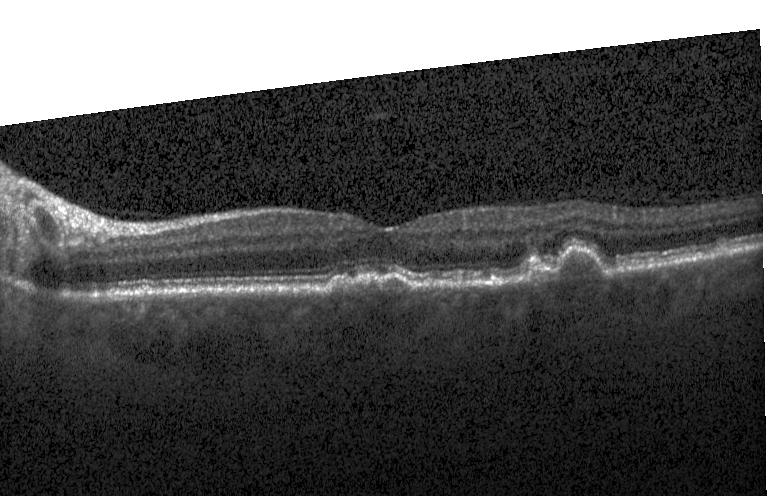 OCT B-scan; spectral-domain OCT — The scan shows sub-RPE drusenoid deposits.